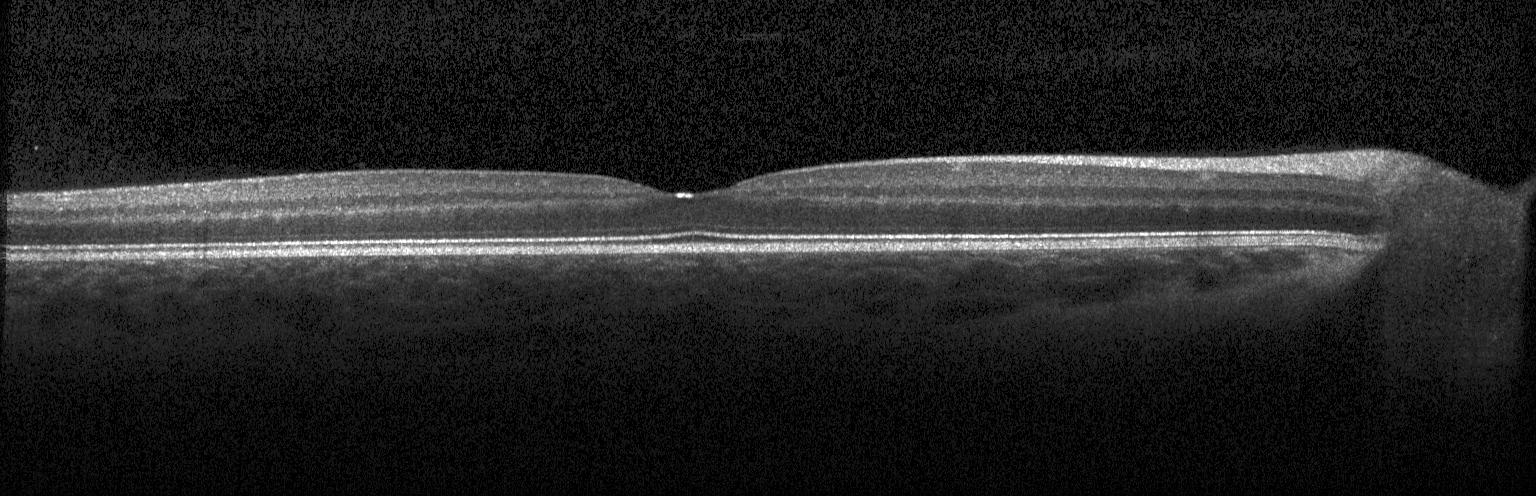

SD-OCT; centered on the fovea; optical coherence tomography scan
Dx: no evidence of choroidal neovascularization, diabetic macular edema, or drusen.